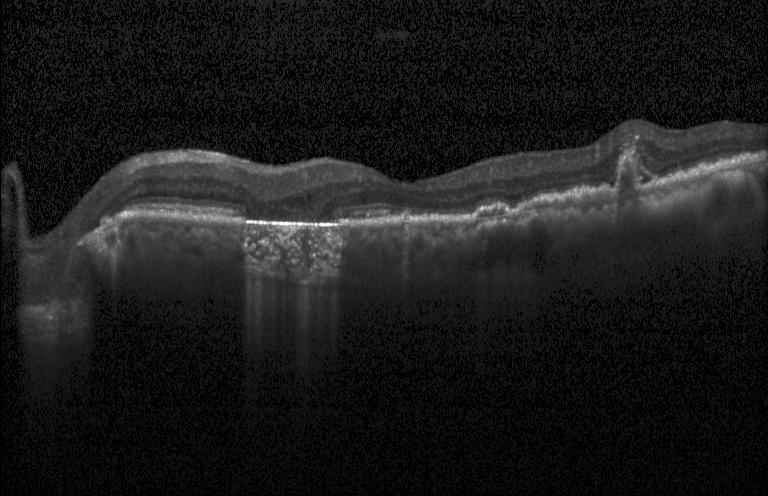 This B-scan demonstrates CNV.